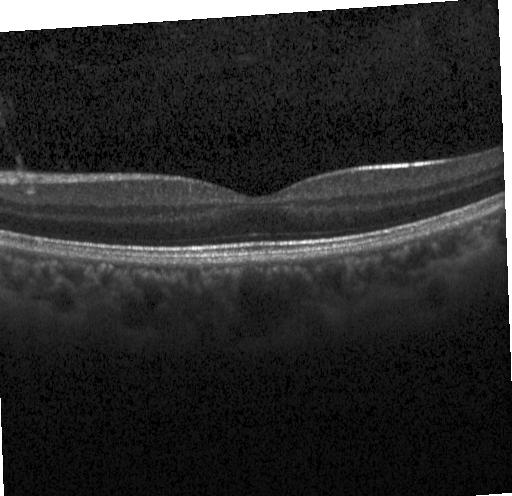
OCT finding: no CNV, no DME, and no drusen.